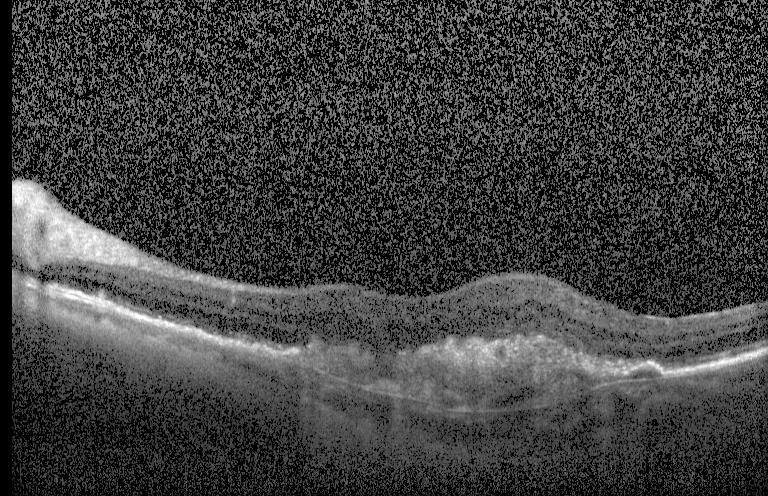 Spectral-domain OCT · OCT line scan · Heidelberg Spectralis.
OCT finding: a choroidal neovascular membrane.